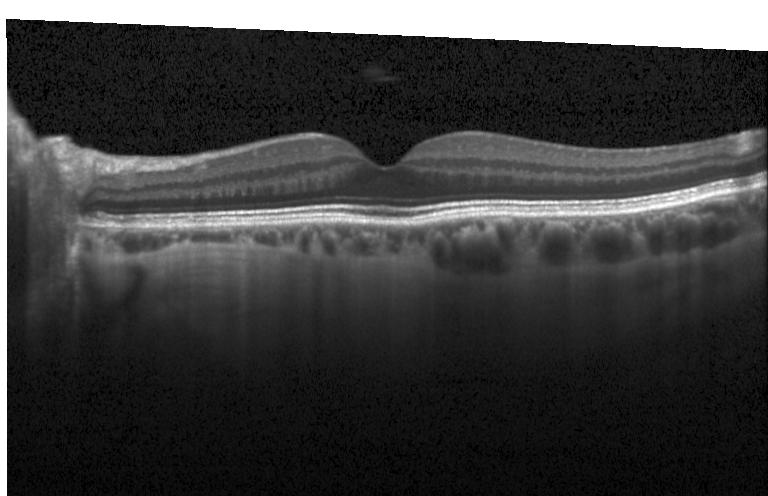 Macular OCT: no CNV, DME, or drusen.